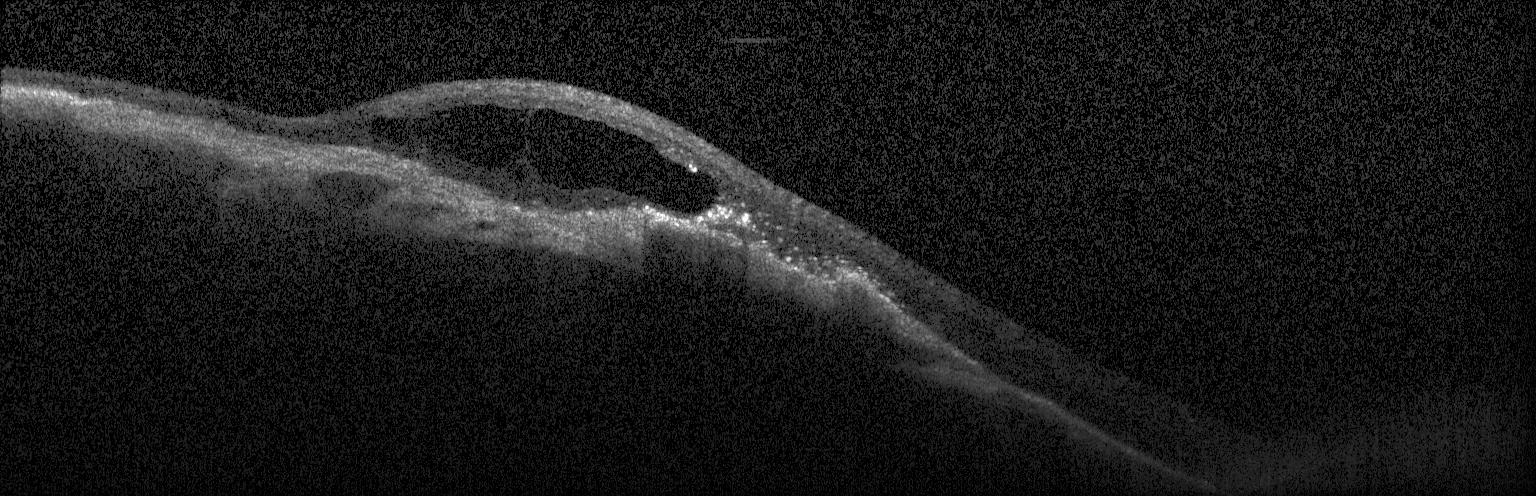 OCT line scan · macular scan · instrument: Heidelberg Spectralis.
Impression: a choroidal neovascular membrane.